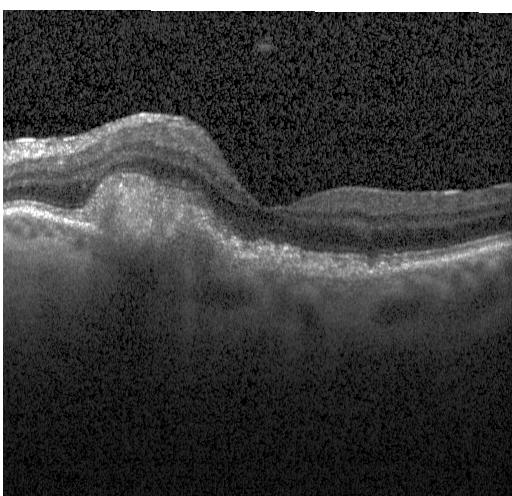 Heidelberg Spectralis OCT system · macular scan · SD-OCT · OCT line scan
Finding: a choroidal neovascular membrane.